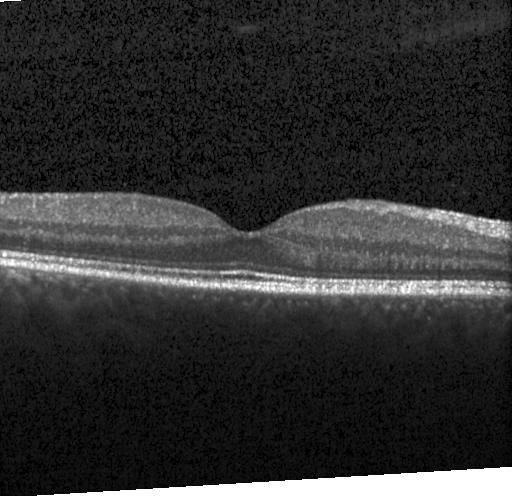
Retinal OCT cross-section — Macular OCT: no CNV, DME, or drusen.